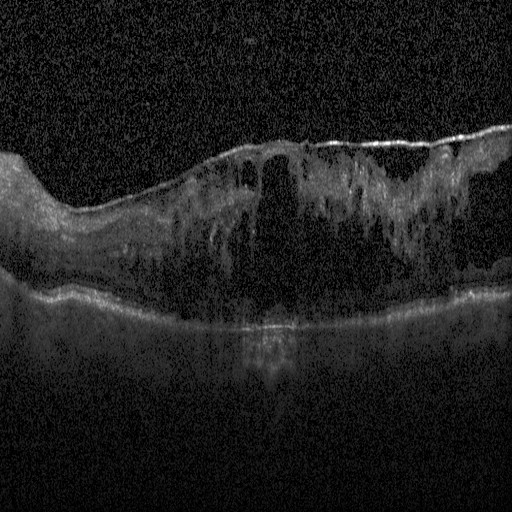
OCT B-scan. Finding: diabetic macular edema.